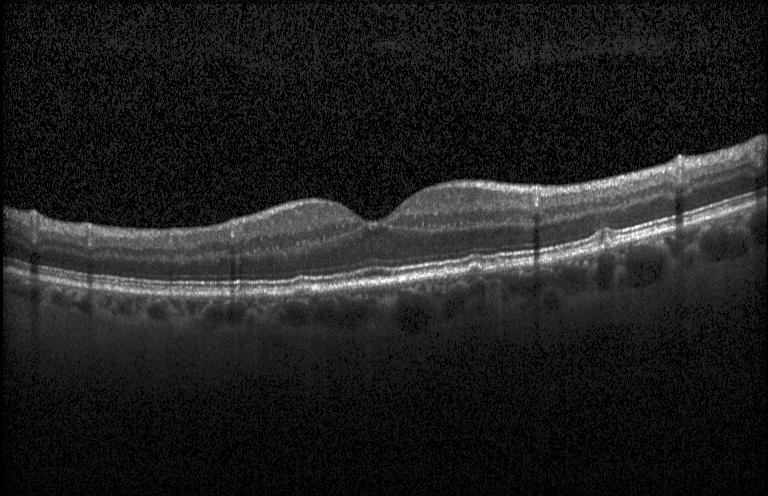

Optical coherence tomography scan — Dx: drusen.